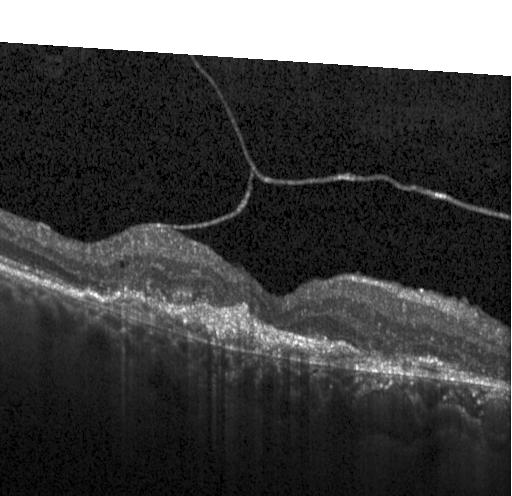
Spectral-domain OCT, through the macula, optical coherence tomography B-scan.
Assessment: a choroidal neovascular membrane.